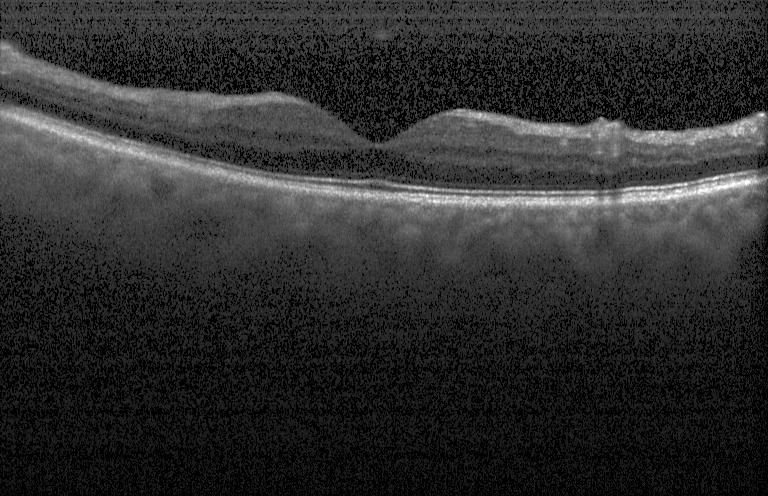
Optical coherence tomography B-scan
Neither choroidal neovascularization, diabetic macular edema, nor drusen.